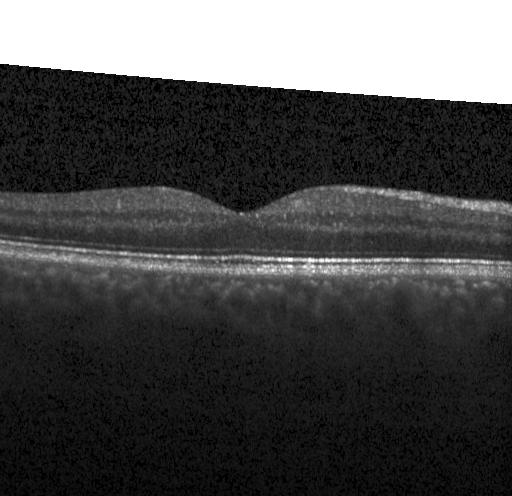
Retinal OCT cross-section showing neither CNV, DME, nor drusen.